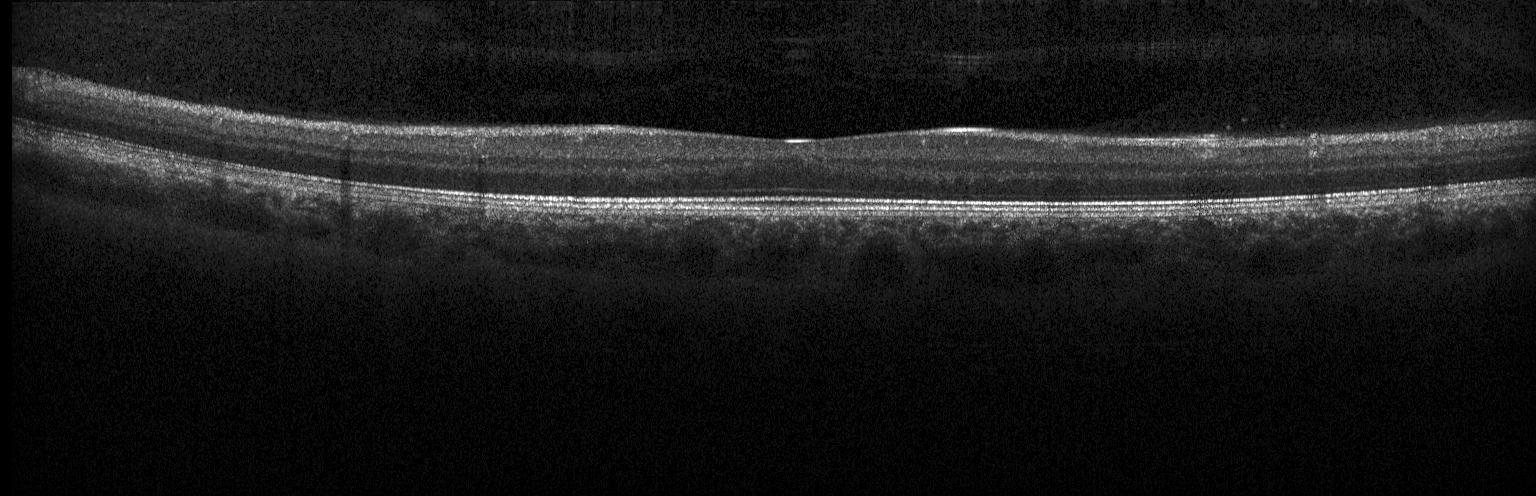 Macular OCT demonstrating no CNV, no DME, and no drusen.